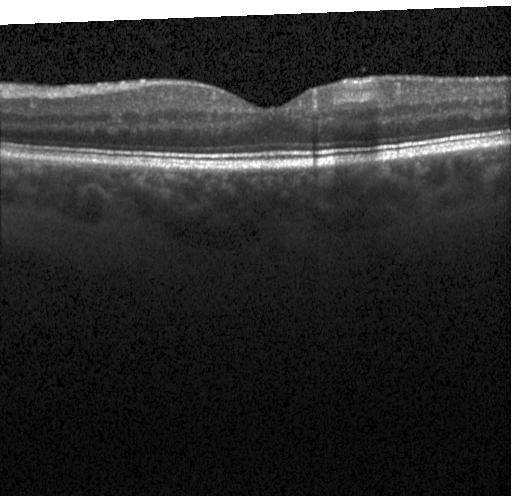

Macular OCT demonstrating no evidence of CNV, DME, or drusen.